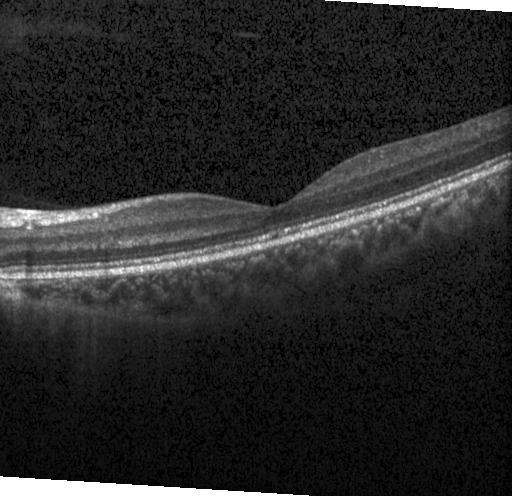
Spectral-domain OCT B-scan: neither choroidal neovascularization, diabetic macular edema, nor drusen.